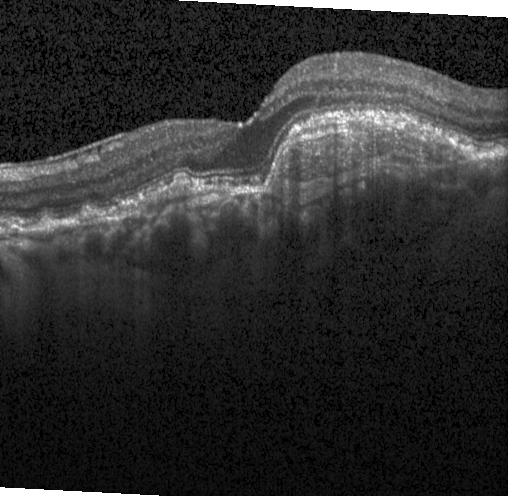

Retinal OCT cross-section · spectral-domain optical coherence tomography · through the macula.
Diagnosis: a choroidal neovascular membrane.